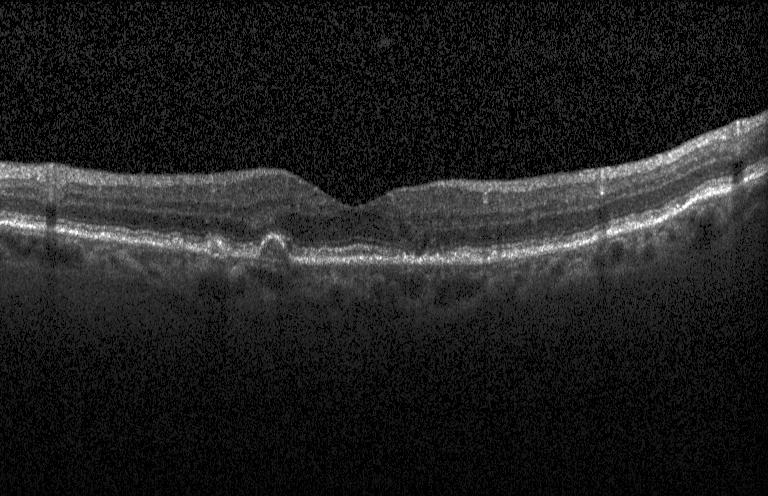

The scan shows multiple drusen.